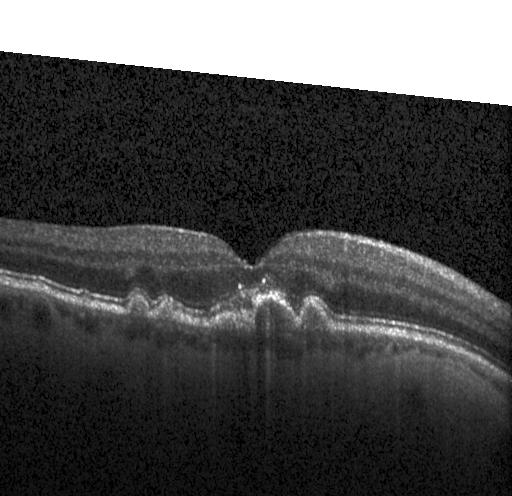
Optical coherence tomography B-scan. Impression: multiple drusen.